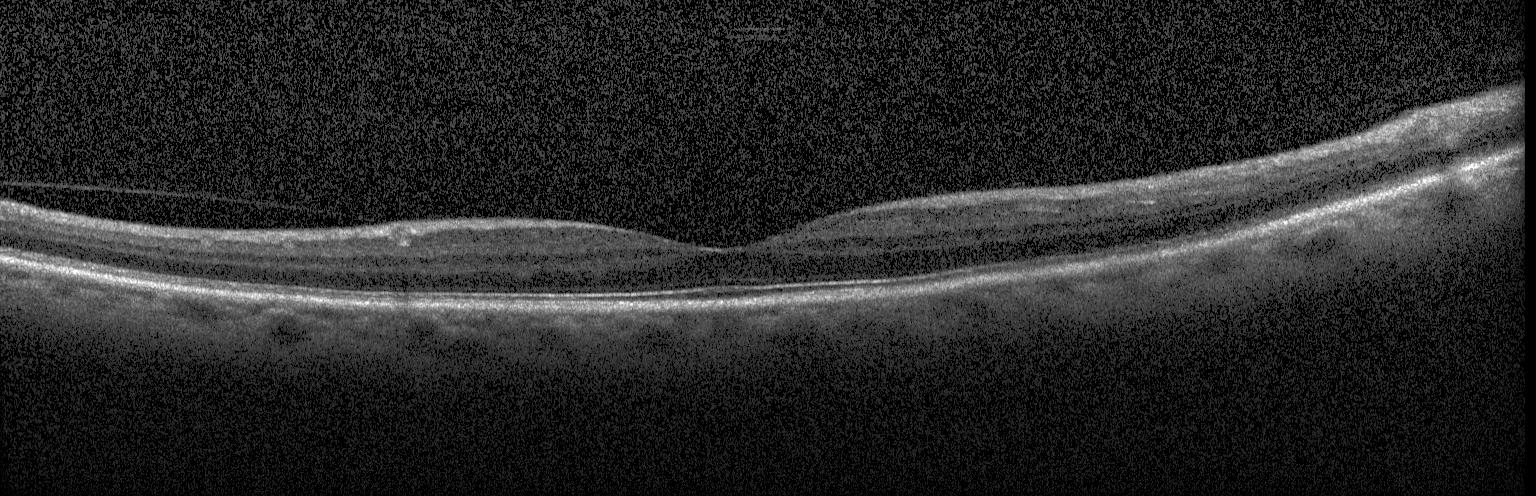 OCT line scan; acquired on a Heidelberg Spectralis.
OCT finding: neither CNV, DME, nor drusen.